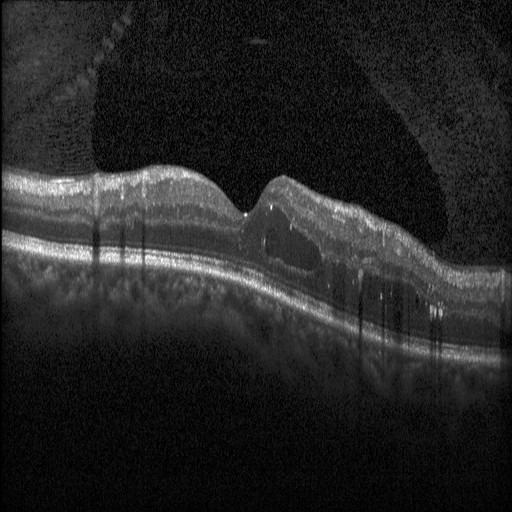

Diabetic macular edema.